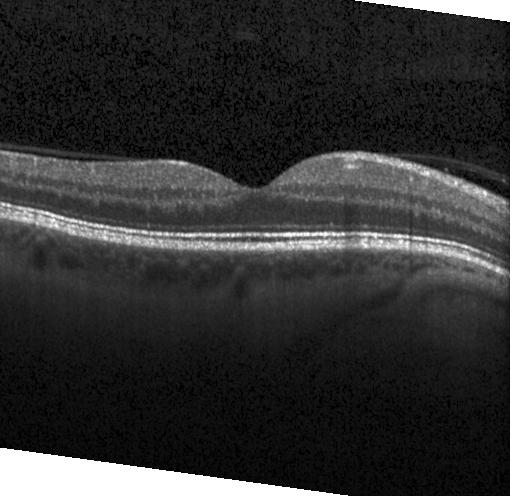

Spectral-domain OCT; OCT B-scan.
This B-scan demonstrates no evidence of choroidal neovascularization, diabetic macular edema, or drusen.